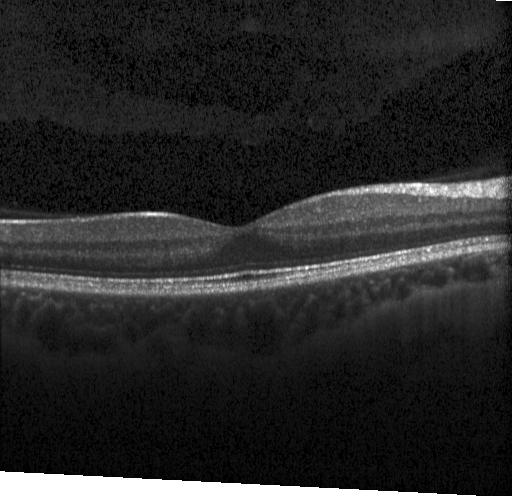

Spectral-domain optical coherence tomography; fovea-centered; OCT B-scan; Heidelberg Spectralis. Impression: no choroidal neovascularization, diabetic macular edema, or drusen.